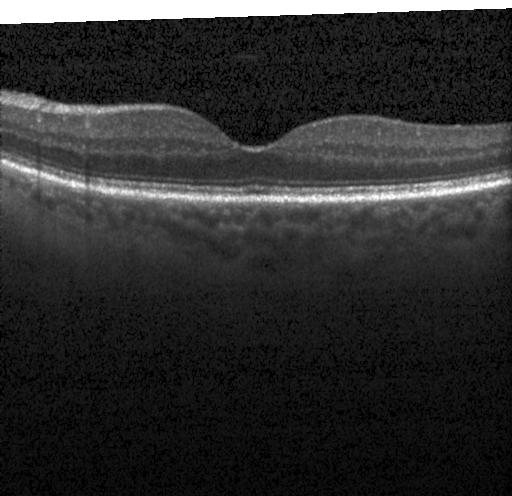

Retinal OCT cross-section.
No evidence of choroidal neovascularization, diabetic macular edema, or drusen.